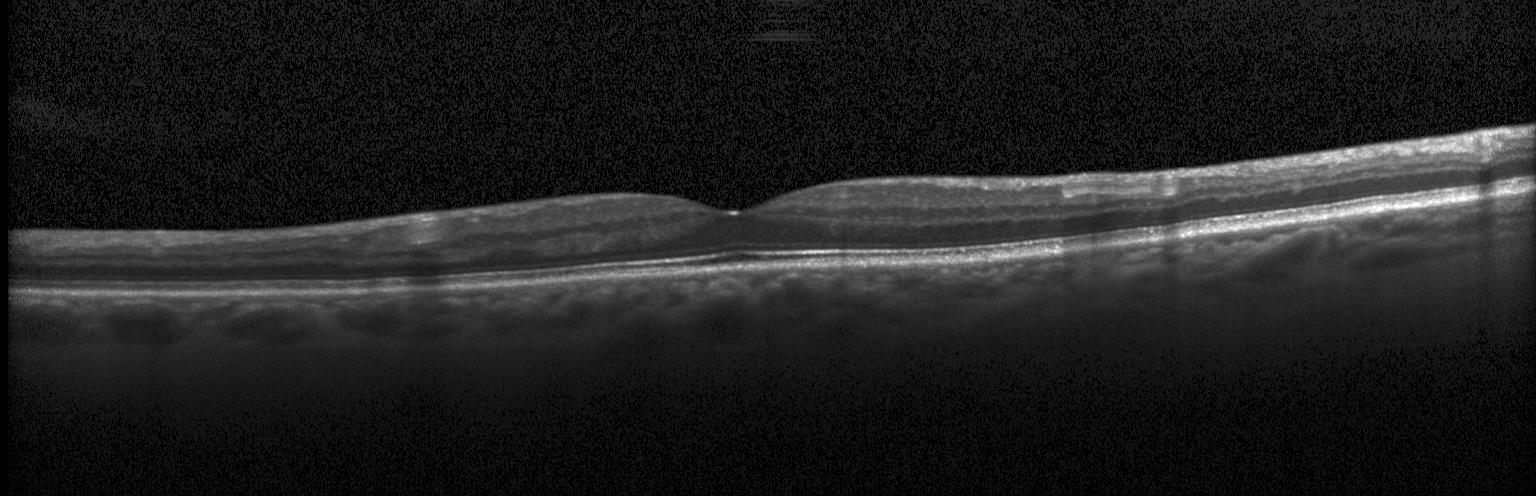
Neither choroidal neovascularization, diabetic macular edema, nor drusen.